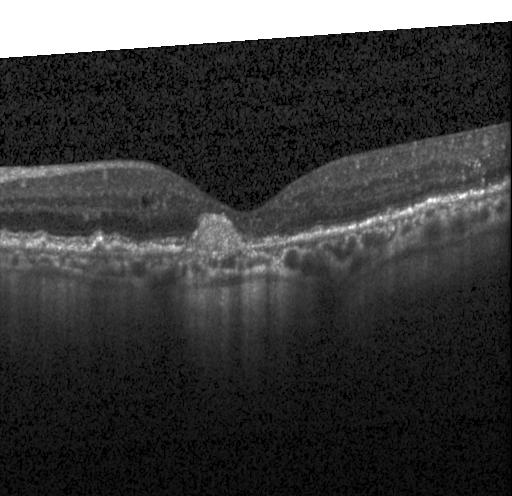 OCT line scan. Macular OCT: CNV.